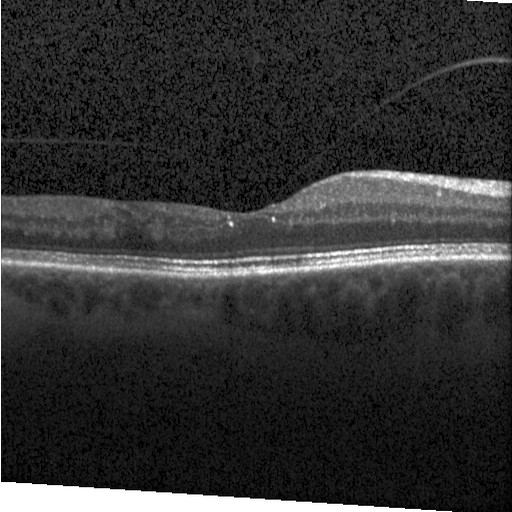

Optical coherence tomography B-scan; spectral-domain OCT.
Impression: diabetic macular edema.